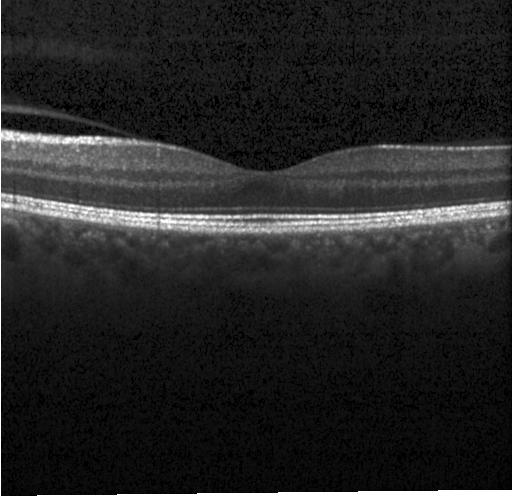

Optical coherence tomography scan.
Diagnosis: no choroidal neovascularization, no diabetic macular edema, and no drusen.